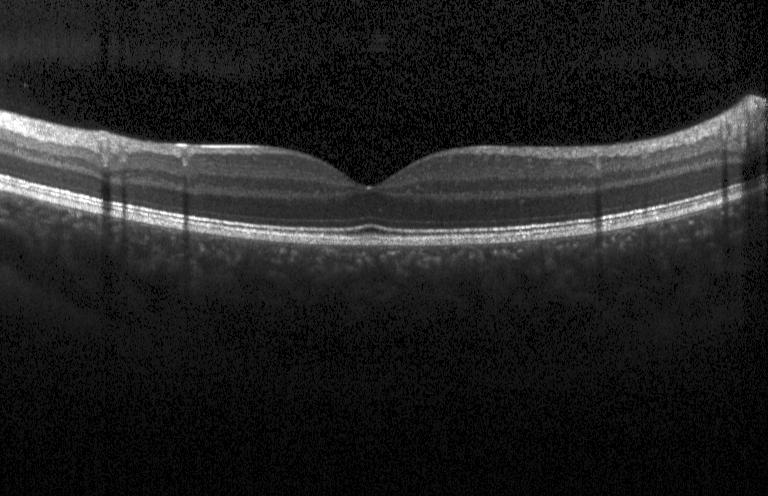

Neither choroidal neovascularization, diabetic macular edema, nor drusen.